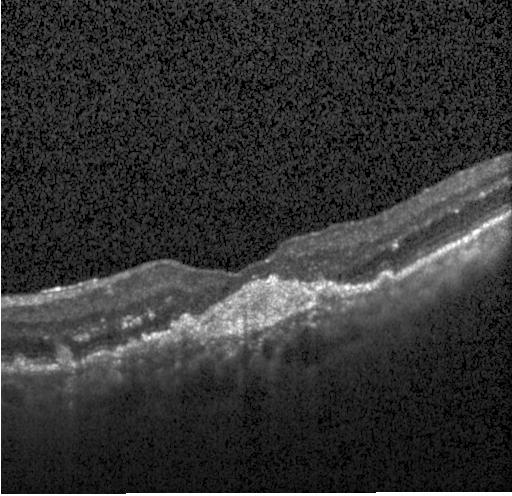
OCT B-scan. Instrument: Heidelberg Spectralis. Fovea-centered. Spectral-domain OCT. This B-scan demonstrates CNV.